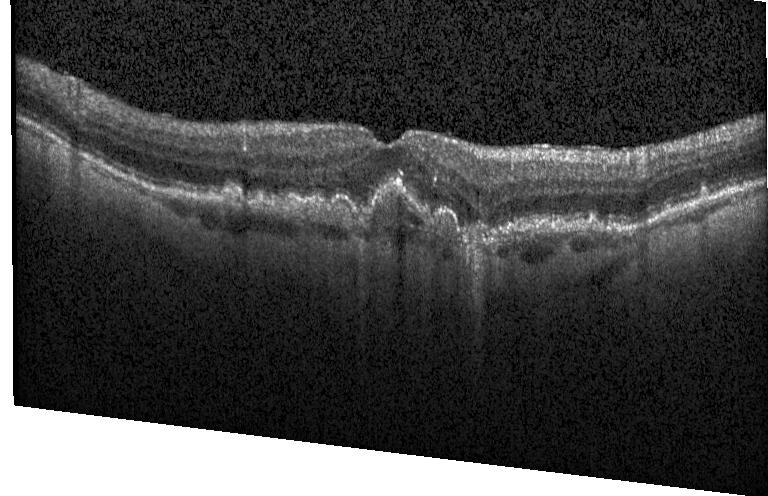
Finding: choroidal neovascularization (CNV).